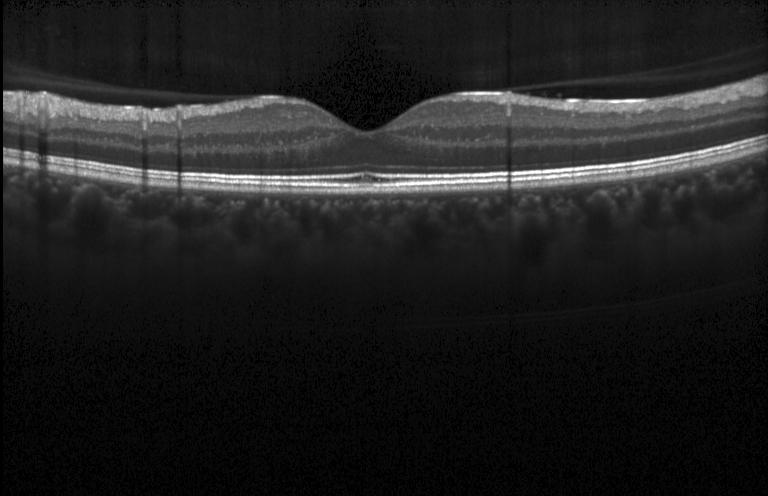
Spectral-domain OCT; optical coherence tomography scan; Heidelberg Spectralis. Impression: no evidence of choroidal neovascularization, diabetic macular edema, or drusen.